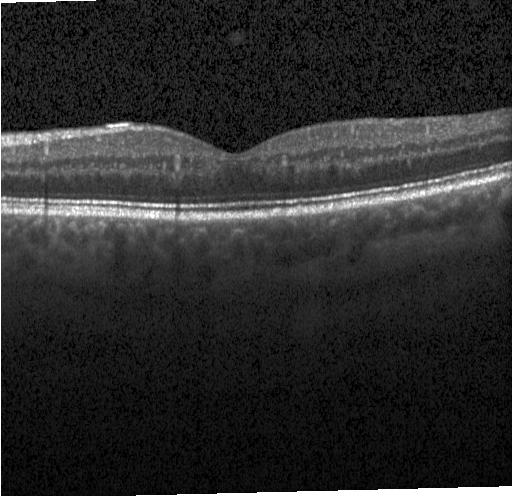 OCT B-scan. SD-OCT. Fovea-centered. Instrument: Heidelberg Spectralis. Finding: no evidence of choroidal neovascularization, diabetic macular edema, or drusen.